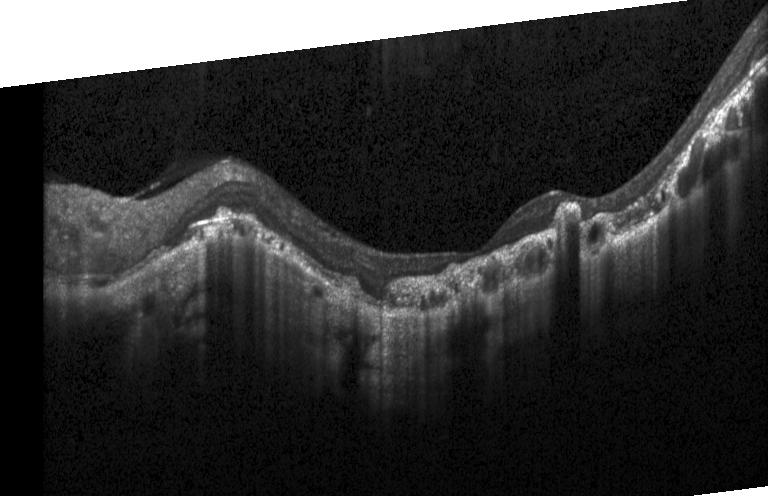
Instrument: Heidelberg Spectralis; OCT line scan; SD-OCT — Assessment: choroidal neovascularization.